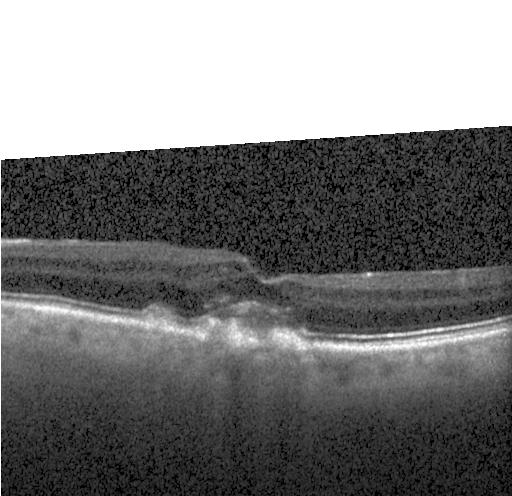
OCT B-scan. Spectral-domain OCT. Instrument: Heidelberg Spectralis. Fovea-centered. A choroidal neovascular membrane.